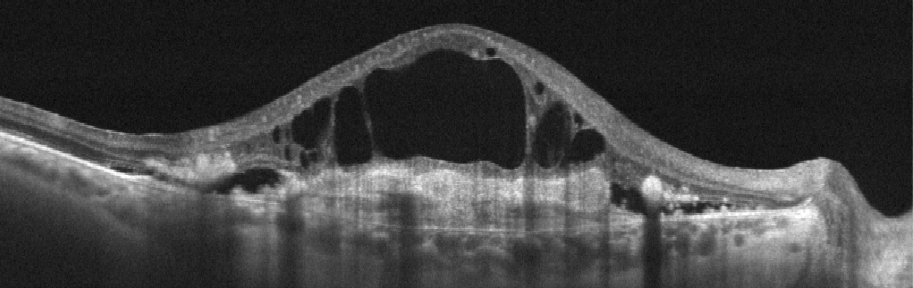
Optical coherence tomography B-scan. Optovue Avanti RTVue XR. Finding: age-related macular degeneration.